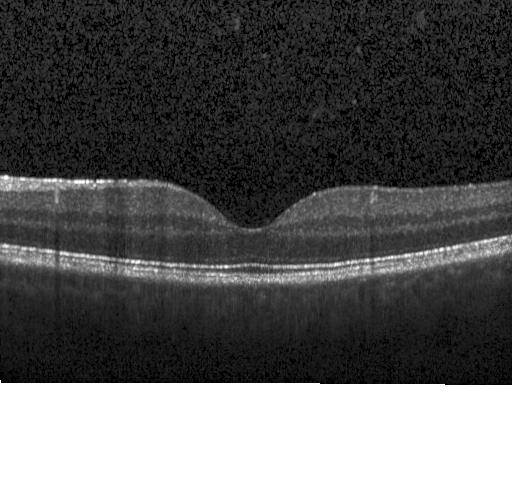
Diagnosis: no CNV, DME, or drusen.